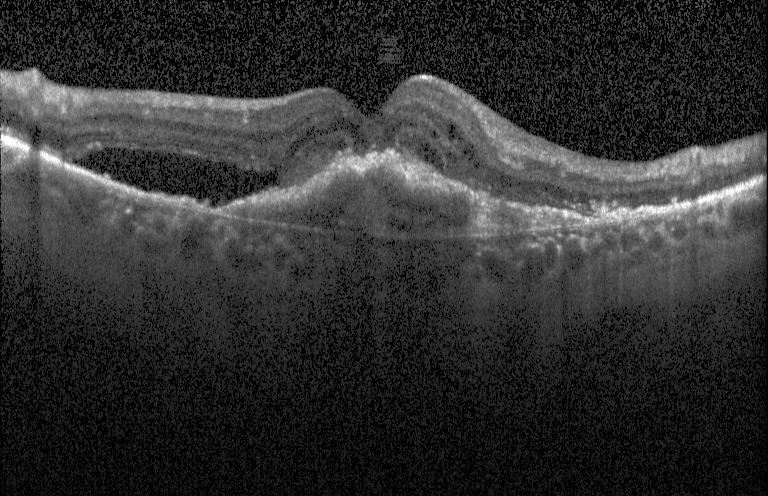

Acquired on a Heidelberg Spectralis · retinal OCT cross-section · SD-OCT — Impression: choroidal neovascularization.